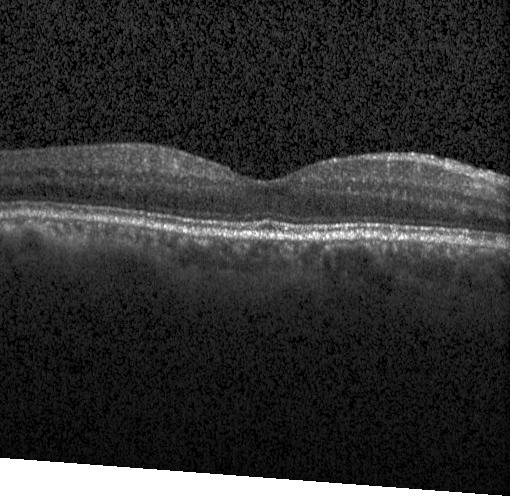

Optical coherence tomography B-scan
Impression: neither CNV, DME, nor drusen.